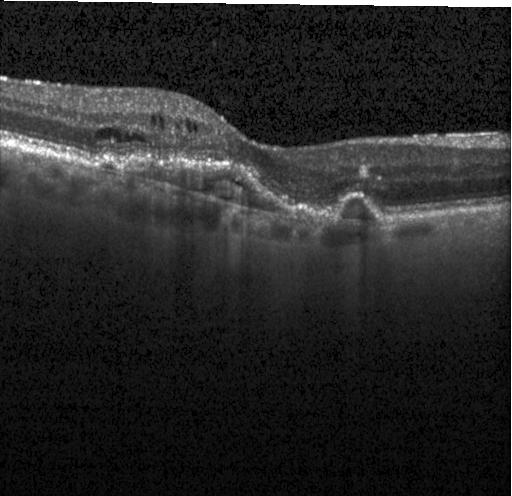 Macular scan; SD-OCT; retinal OCT cross-section; Heidelberg Spectralis
OCT finding: a choroidal neovascular membrane.